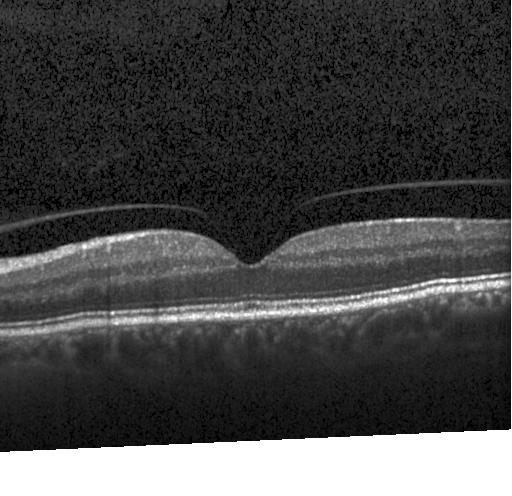
Optical coherence tomography scan.
Macular OCT: no choroidal neovascularization, no diabetic macular edema, and no drusen.